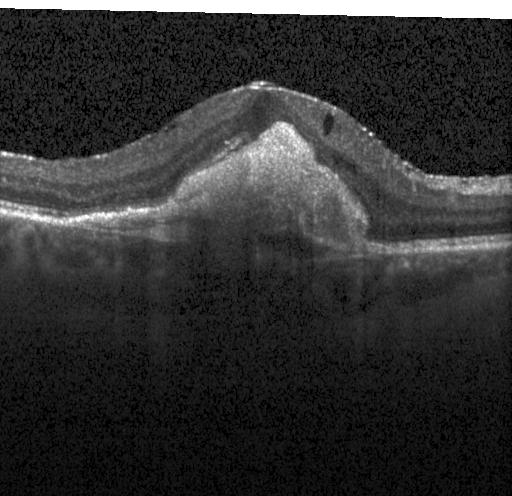
Horizontal scan through the fovea. Retinal OCT B-scan
The scan shows choroidal neovascularization (CNV).